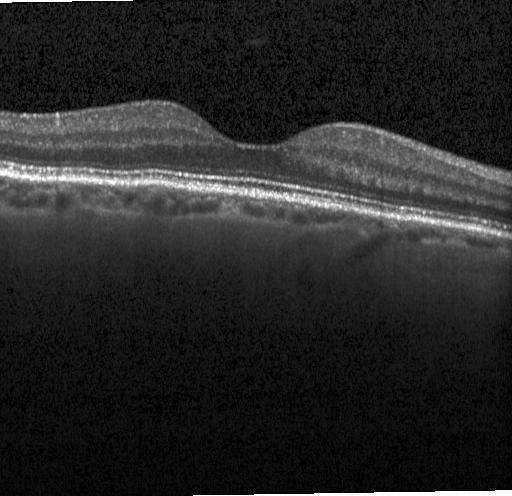
SD-OCT · Heidelberg Spectralis OCT system · OCT line scan.
OCT finding: no choroidal neovascularization, no diabetic macular edema, and no drusen.